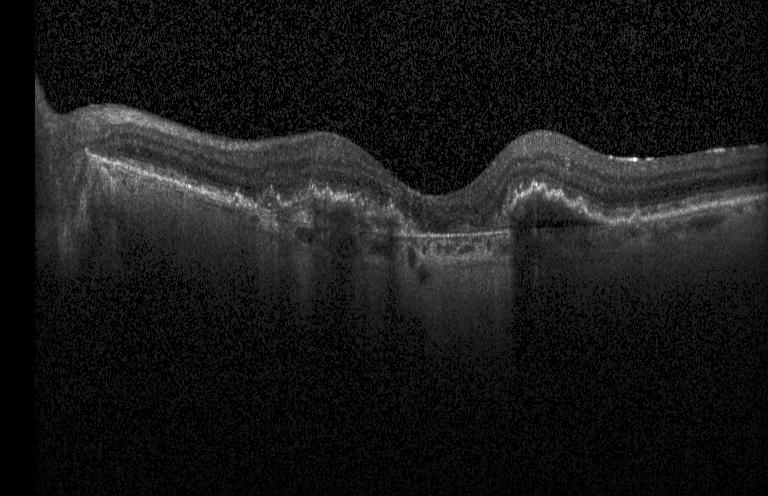 OCT B-scan showing choroidal neovascularization.